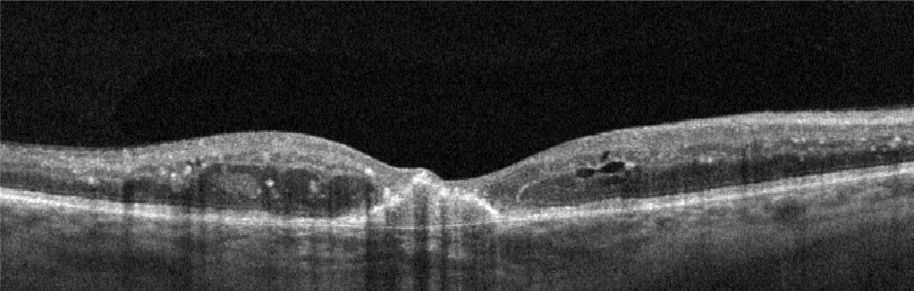
OCT B-scan.
Finding: AMD.